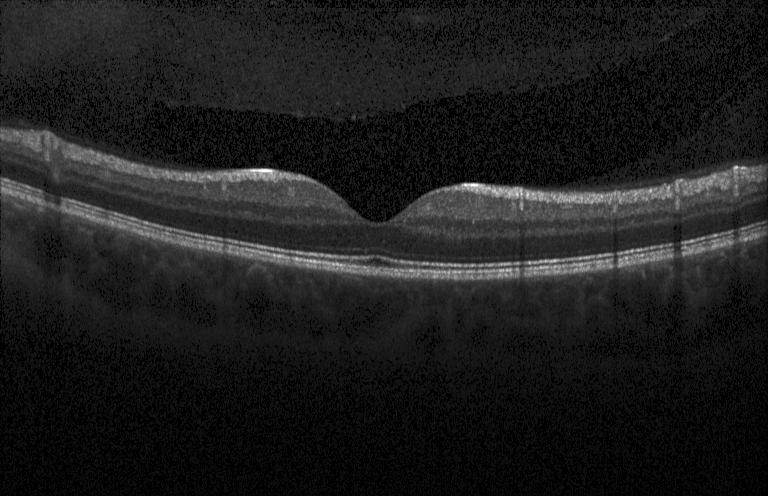

Retinal OCT cross-section · centered on the fovea
No choroidal neovascularization, diabetic macular edema, or drusen.